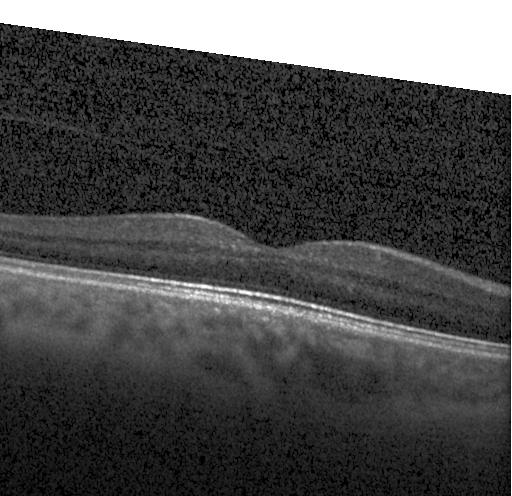

OCT B-scan.
Diagnosis: no choroidal neovascularization, no diabetic macular edema, and no drusen.